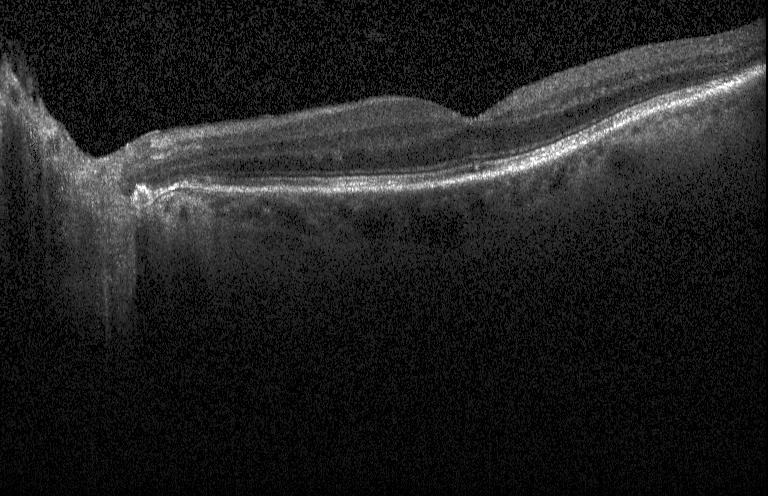

Retinal OCT B-scan
OCT finding: no evidence of choroidal neovascularization, diabetic macular edema, or drusen.